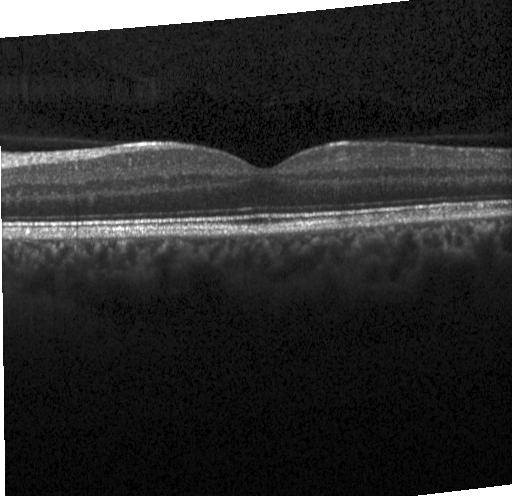
OCT B-scan.
Assessment: no choroidal neovascularization, diabetic macular edema, or drusen.